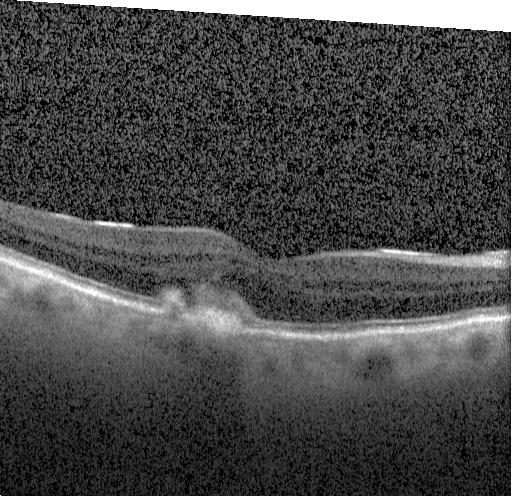
Retinal OCT cross-section · through the macula
Impression: a choroidal neovascular membrane.